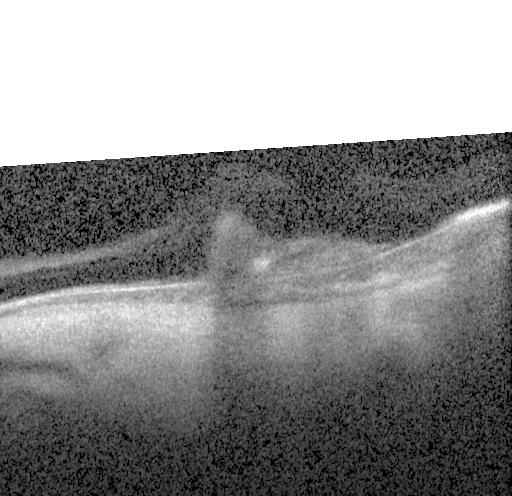
Macular OCT demonstrating a choroidal neovascular membrane.